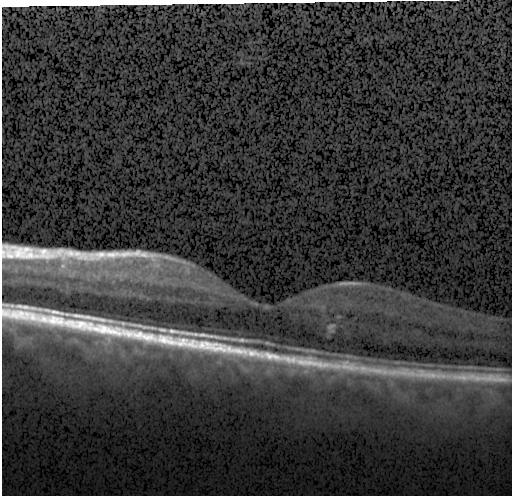 Retinal OCT B-scan · Heidelberg Spectralis · SD-OCT
Assessment: no evidence of CNV, DME, or drusen.